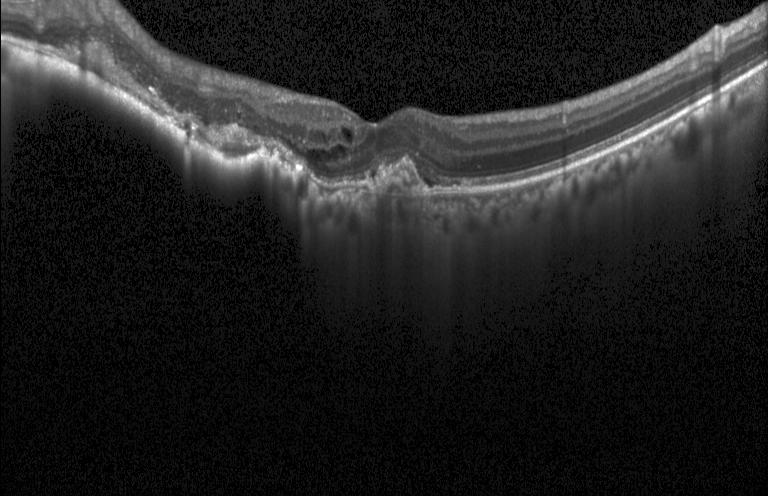
Assessment: a choroidal neovascular membrane.